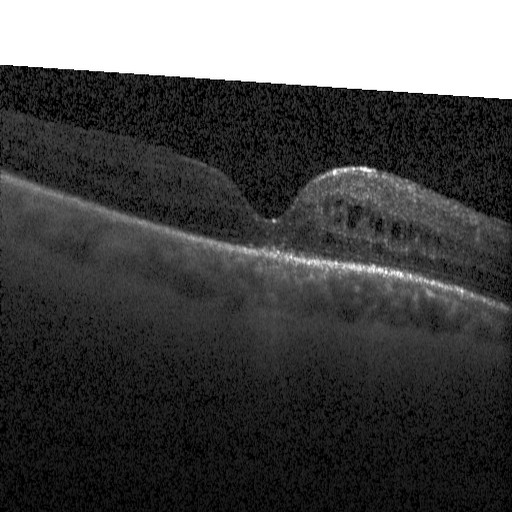
The scan shows diabetic macular edema.